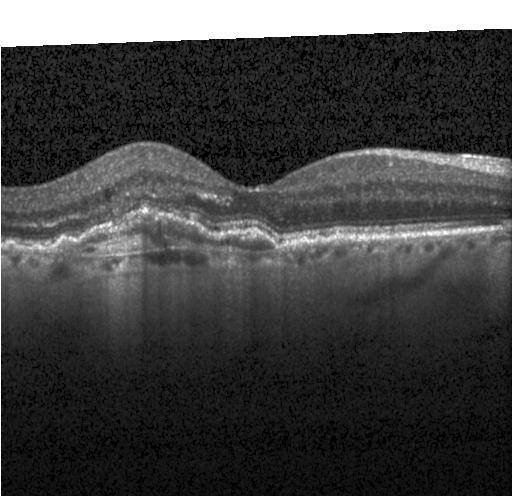

OCT scan showing a choroidal neovascular membrane.